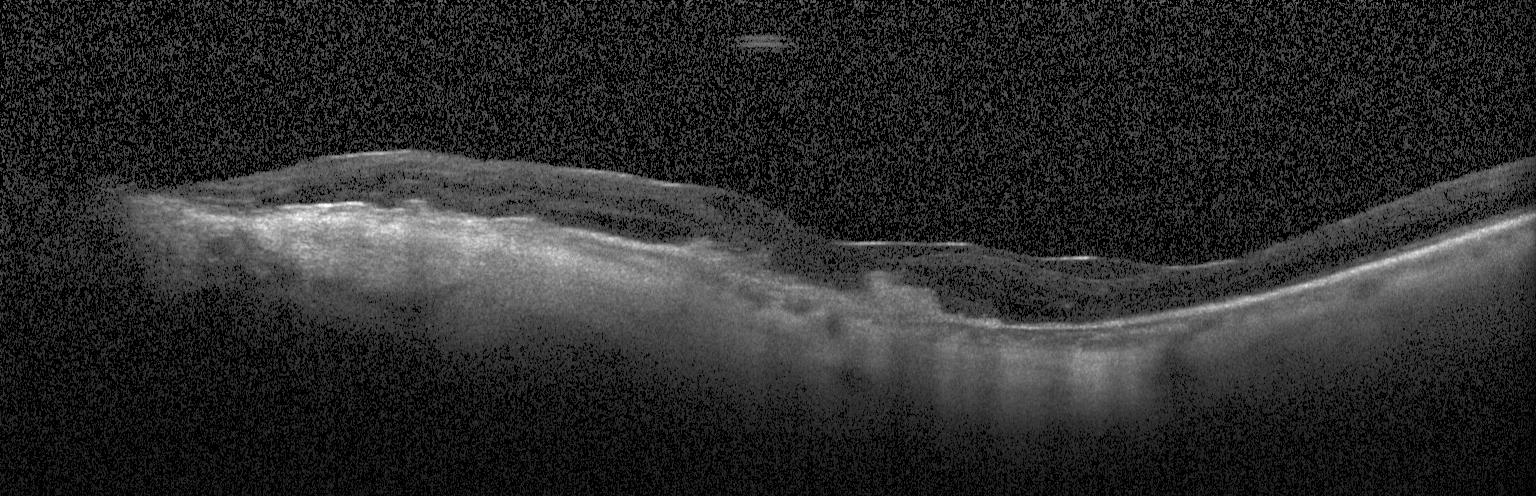 Finding: a choroidal neovascular membrane.